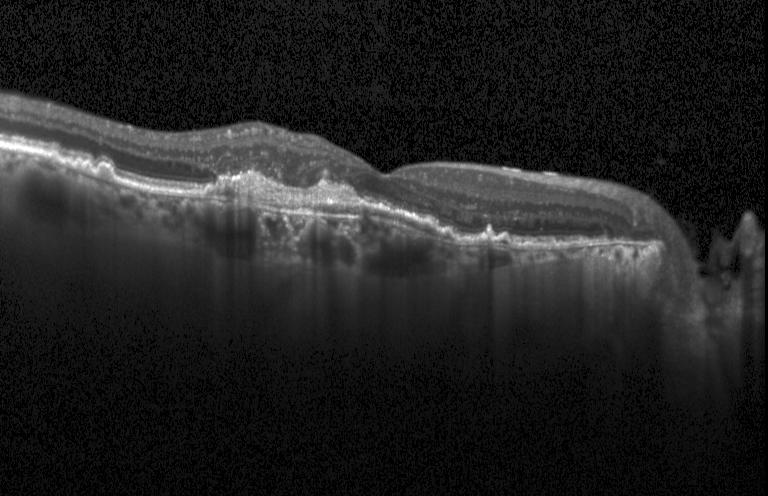 The scan shows choroidal neovascularization (CNV).